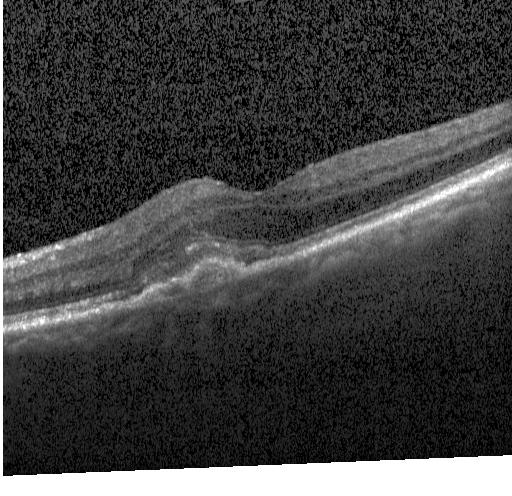

Optical coherence tomography scan
Impression: choroidal neovascularization.